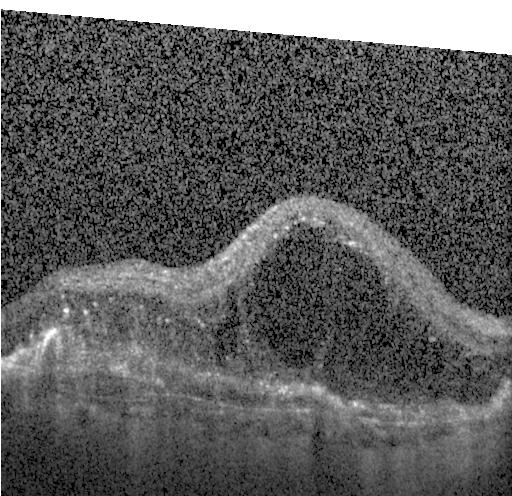

Acquired on a Heidelberg Spectralis; OCT B-scan — Finding: a choroidal neovascular membrane.